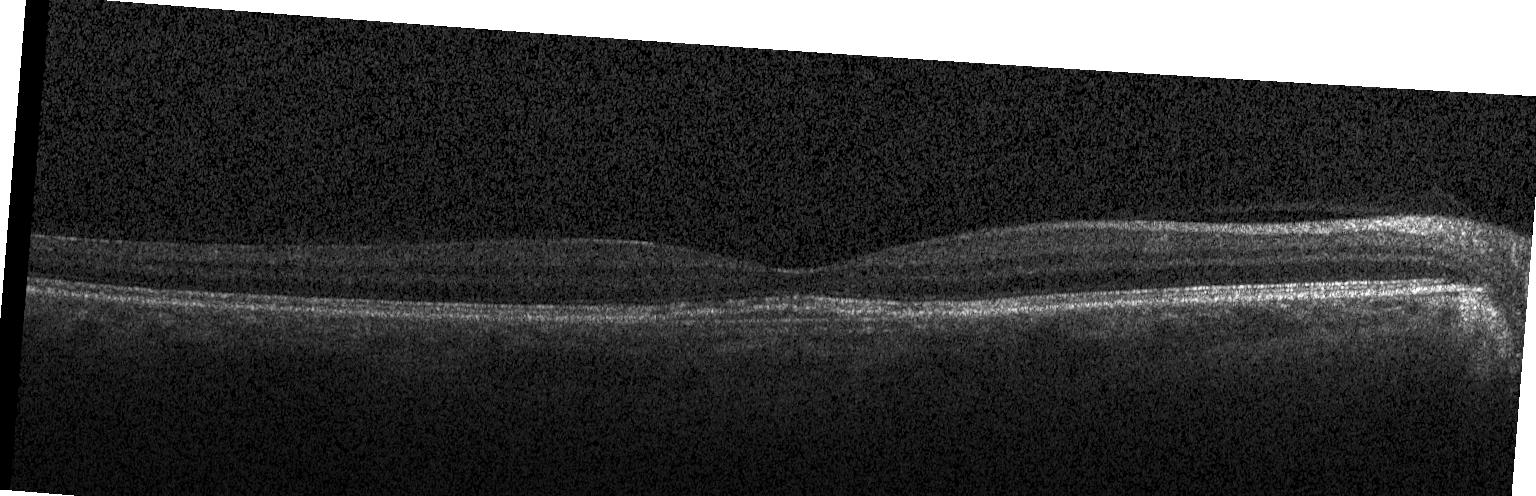
Diagnosis: choroidal neovascularization.